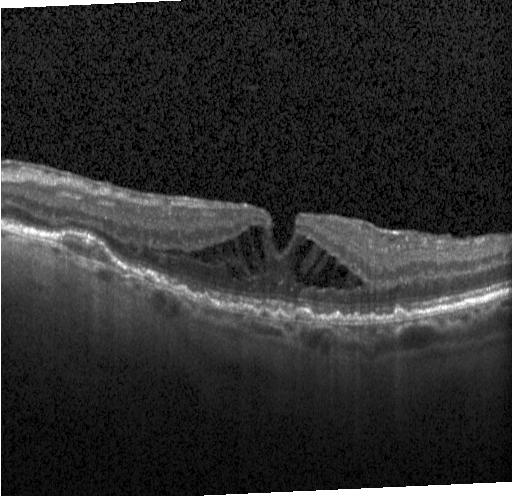

Impression: DME.